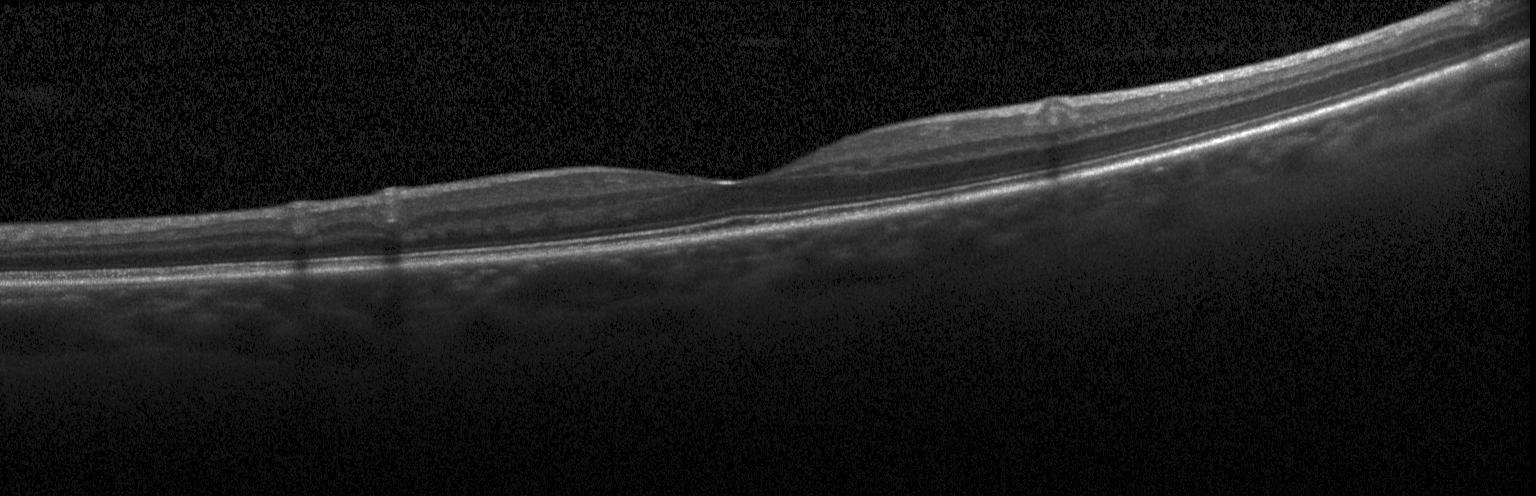
Finding: no choroidal neovascularization, diabetic macular edema, or drusen.